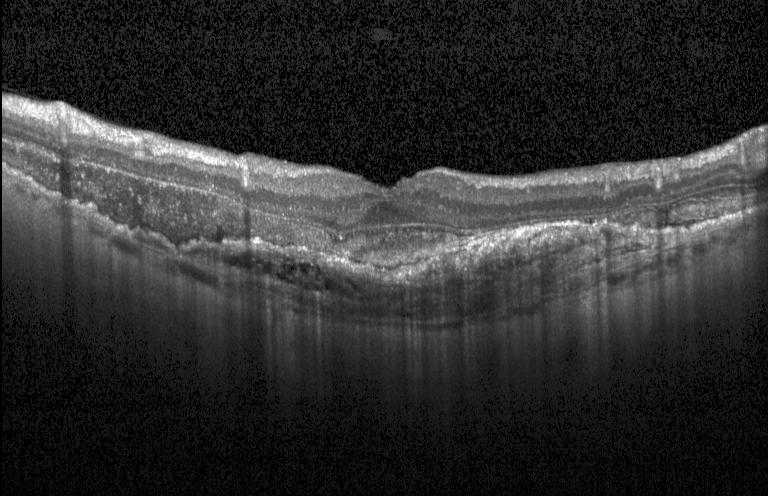
Choroidal neovascularization.